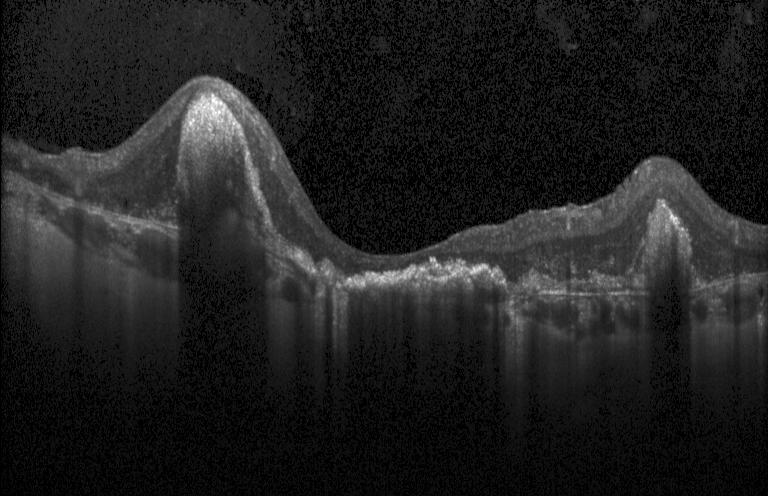 Spectral-domain optical coherence tomography. OCT line scan.
Finding: a choroidal neovascular membrane.